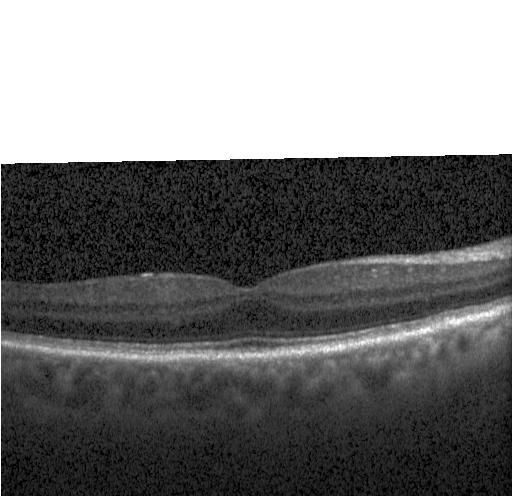 Through the macula. Optical coherence tomography scan. SD-OCT — The scan shows no CNV, DME, or drusen.